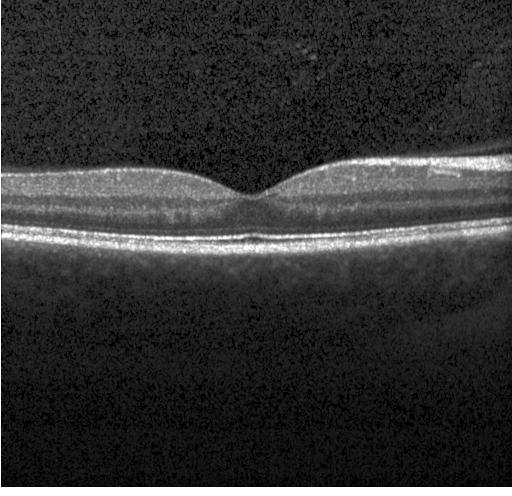

Finding: no CNV, no DME, and no drusen.